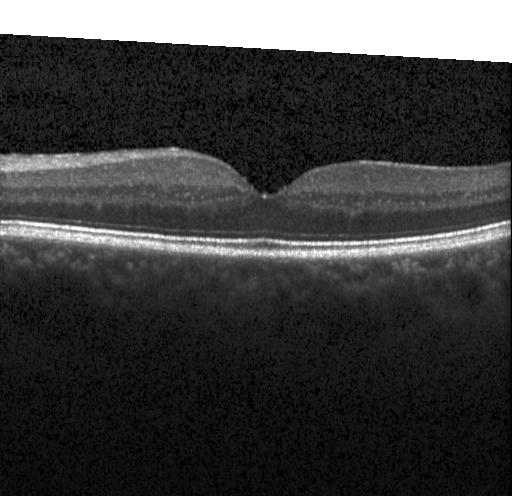
Retinal OCT B-scan, instrument: Heidelberg Spectralis, fovea-centered.
Assessment: no CNV, DME, or drusen.